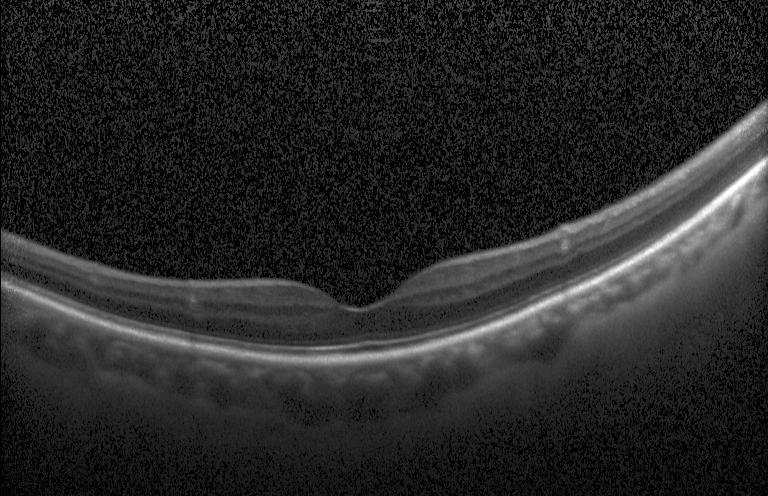
OCT line scan, through the macula, spectral-domain OCT, instrument: Heidelberg Spectralis. Macular OCT: no choroidal neovascularization, no diabetic macular edema, and no drusen.